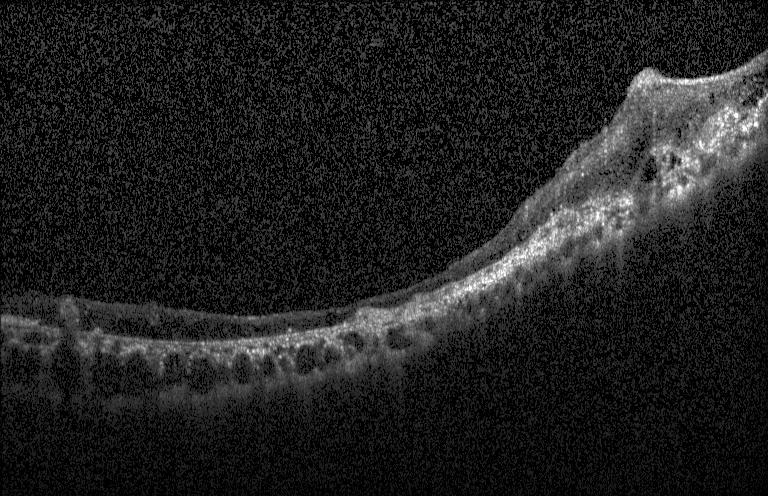

Impression: choroidal neovascularization (CNV).